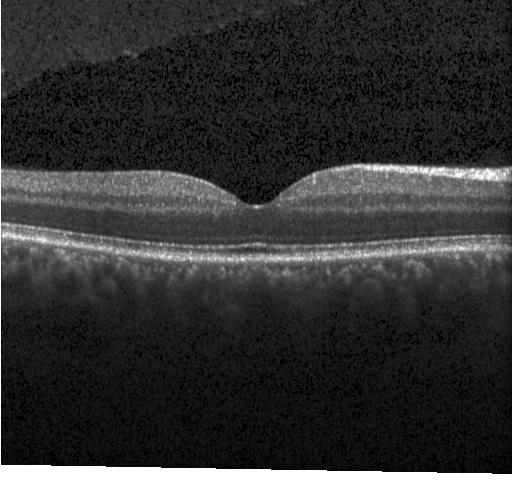

OCT scan showing no choroidal neovascularization, diabetic macular edema, or drusen.